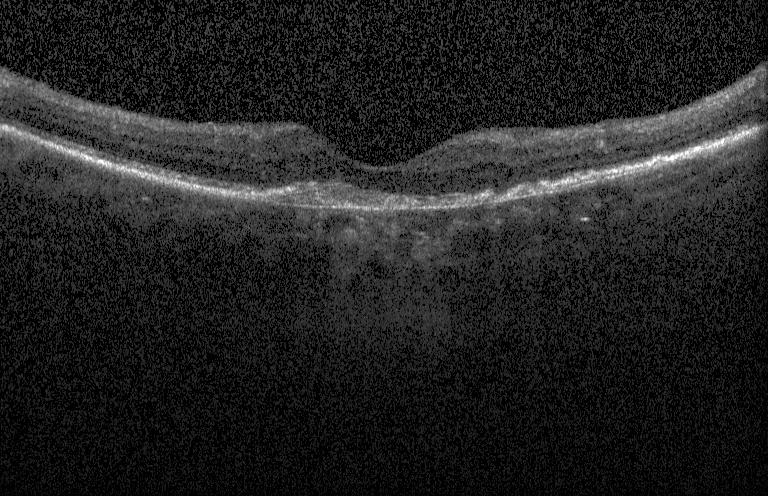

Spectral-domain optical coherence tomography; retinal OCT cross-section; macular scan.
CNV.